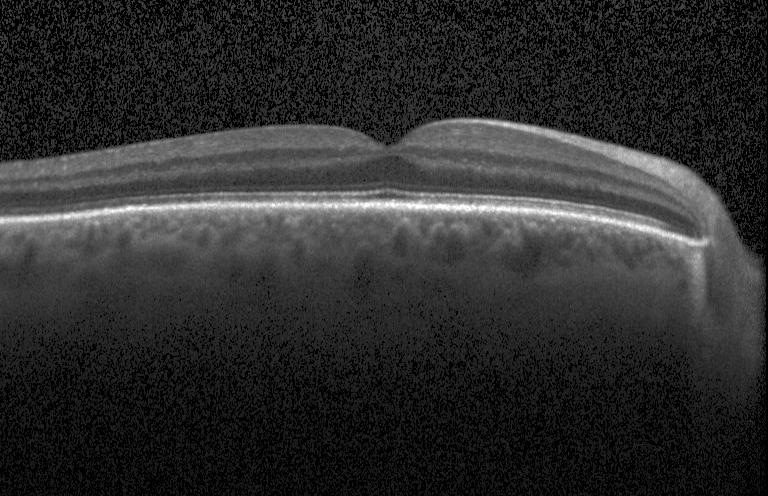
SD-OCT; optical coherence tomography scan. OCT finding: neither CNV, DME, nor drusen.